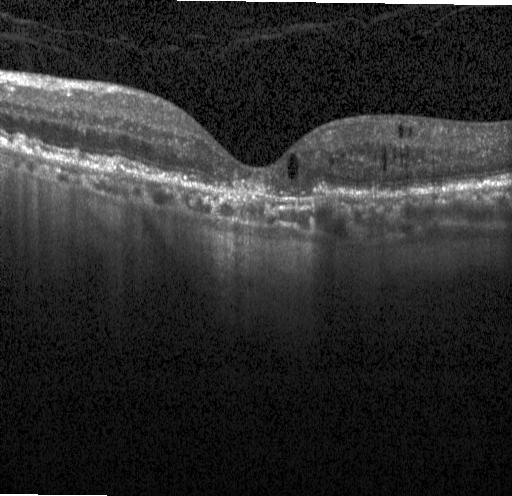
Retinal OCT B-scan · fovea-centered — A choroidal neovascular membrane.